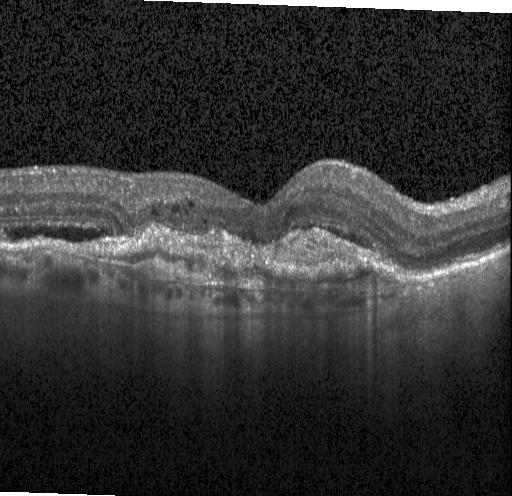

SD-OCT, Heidelberg Spectralis, through the macula, OCT B-scan.
Diagnosis: choroidal neovascularization (CNV).